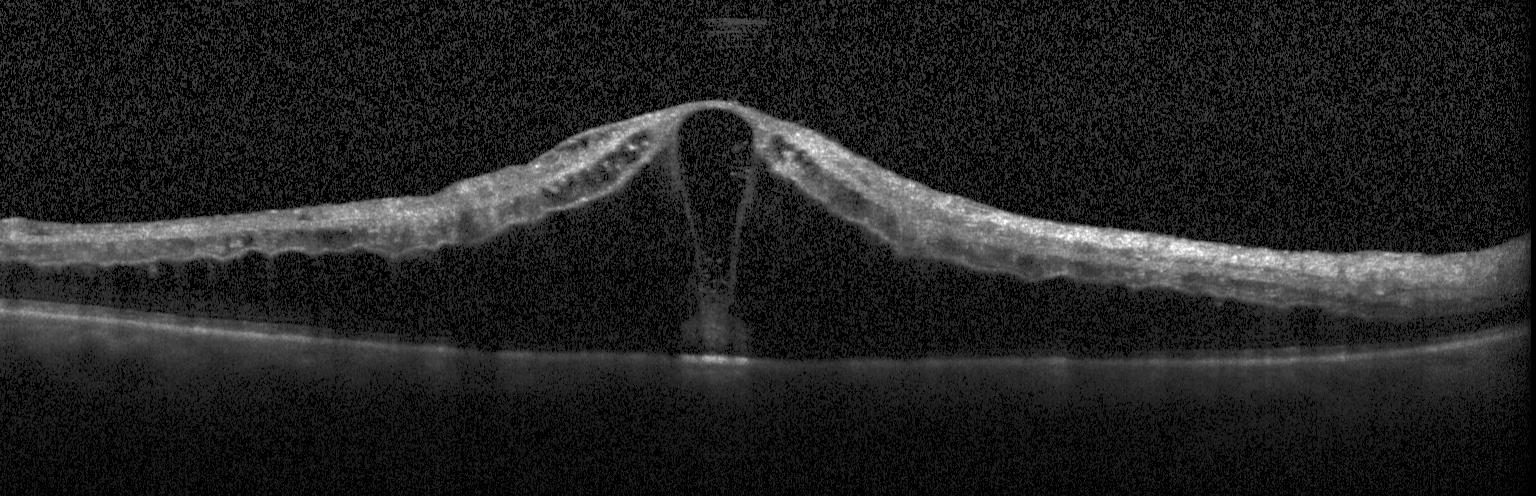 OCT B-scan; Heidelberg Spectralis OCT system — OCT finding: DME.